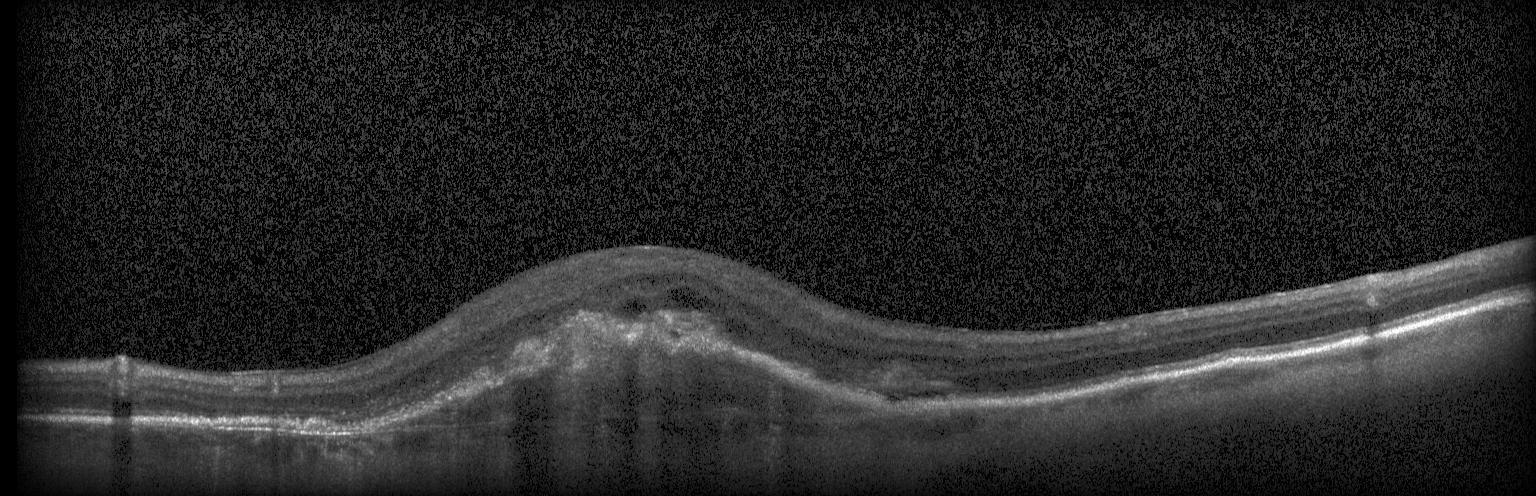
Finding: choroidal neovascularization.